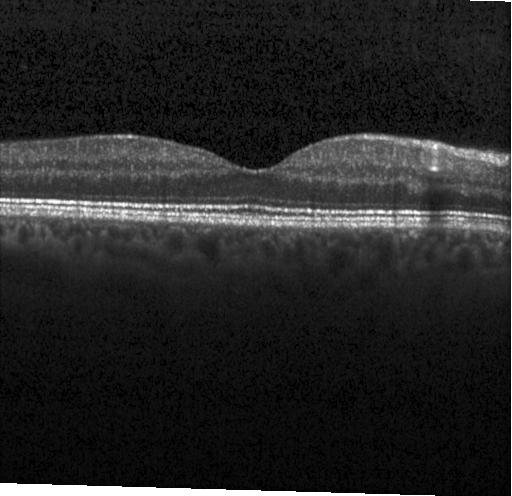
Optical coherence tomography scan — Finding: no CNV, no DME, and no drusen.